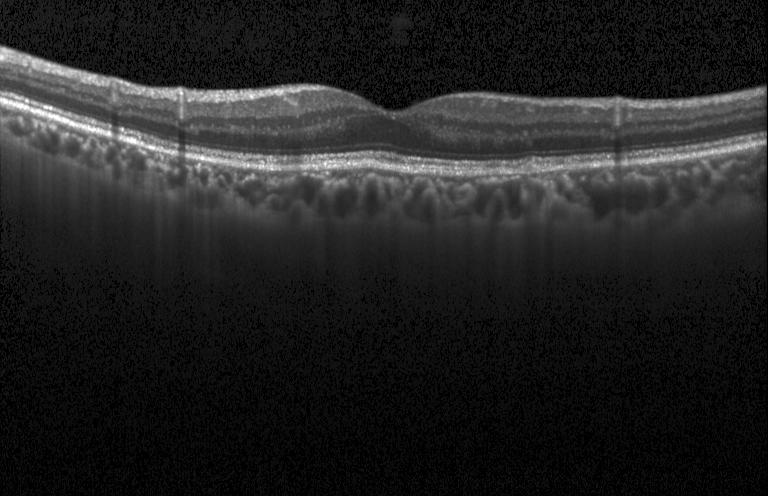
Retinal OCT cross-section. Macular scan. Heidelberg Spectralis
Diagnosis: neither choroidal neovascularization, diabetic macular edema, nor drusen.